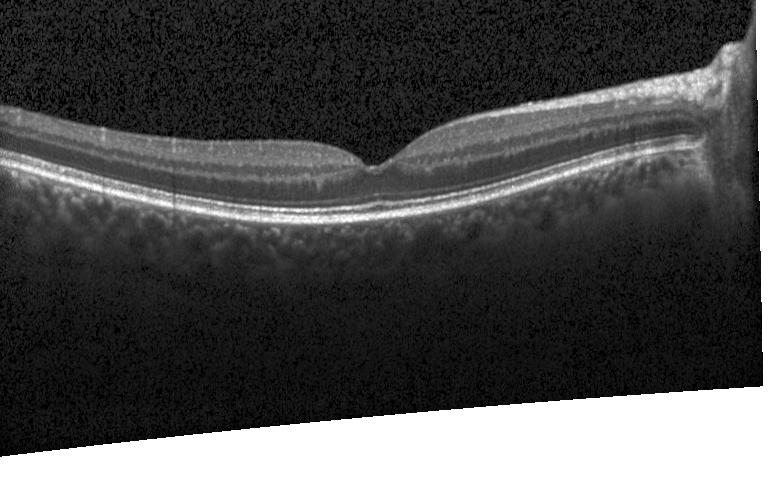
Impression: no evidence of choroidal neovascularization, diabetic macular edema, or drusen.